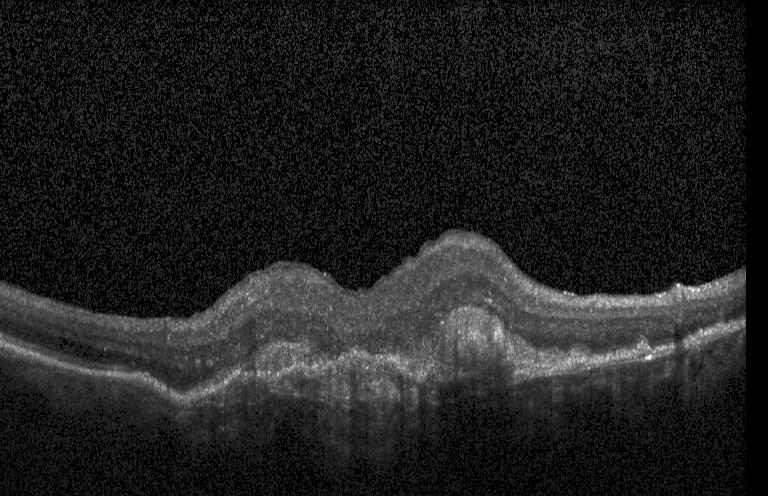
Finding: choroidal neovascularization (CNV).